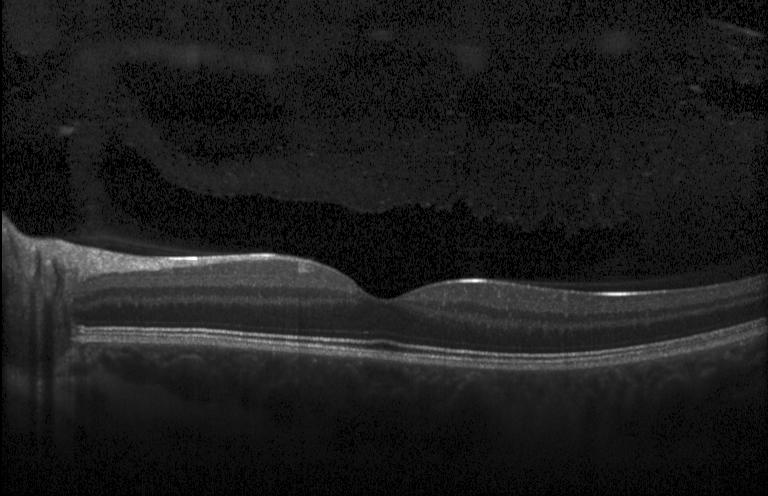 Impression: no evidence of choroidal neovascularization, diabetic macular edema, or drusen.